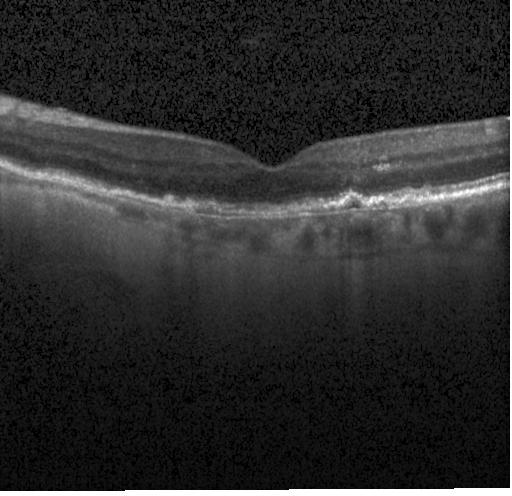 OCT B-scan showing drusen.